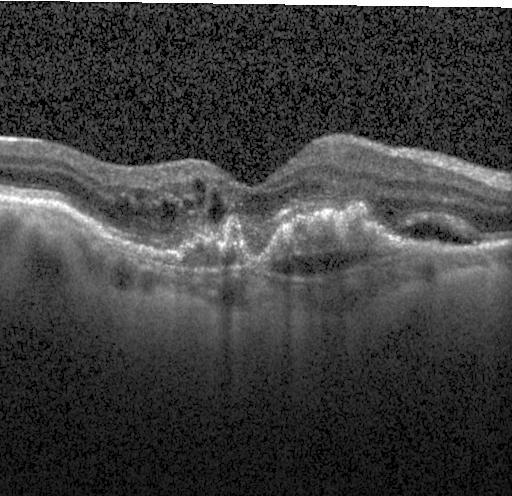

Retinal OCT cross-section showing choroidal neovascularization (CNV).